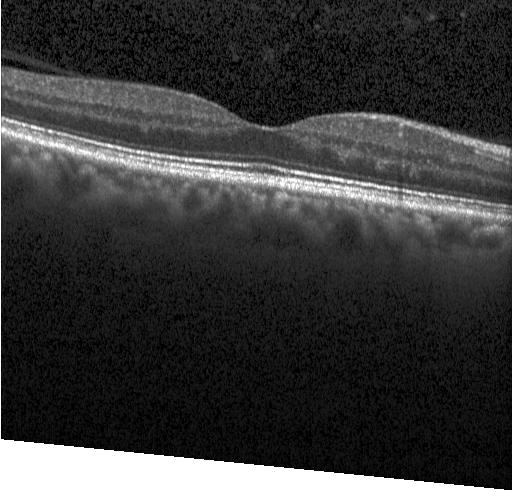

Instrument: Heidelberg Spectralis; retinal OCT cross-section; spectral-domain OCT — This B-scan demonstrates no choroidal neovascularization, diabetic macular edema, or drusen.